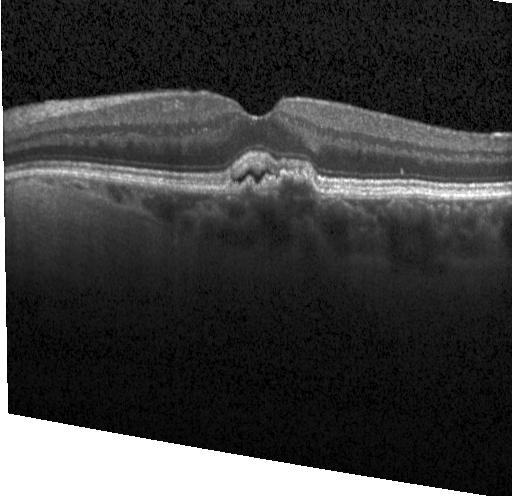

OCT line scan · acquired on a Heidelberg Spectralis
Dx: choroidal neovascularization (CNV).